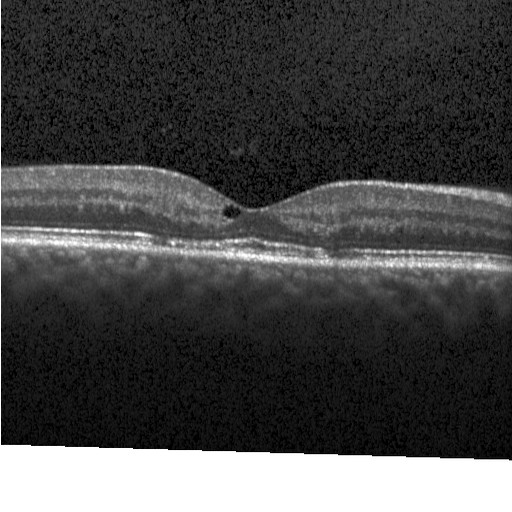 Assessment: DME.